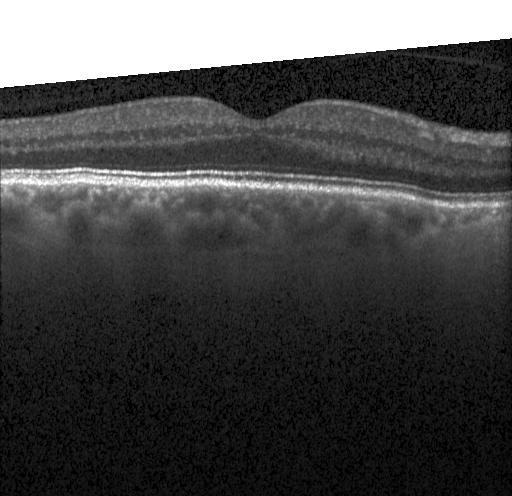

Horizontal scan through the fovea. Spectral-domain OCT. OCT B-scan.
Finding: neither CNV, DME, nor drusen.